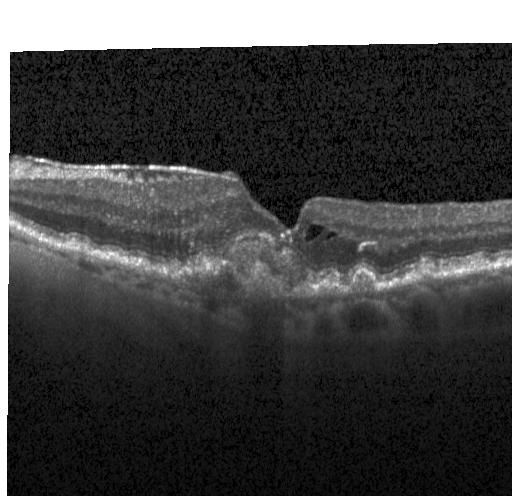

Through the macula · optical coherence tomography scan · spectral-domain optical coherence tomography.
Macular OCT: choroidal neovascularization (CNV).